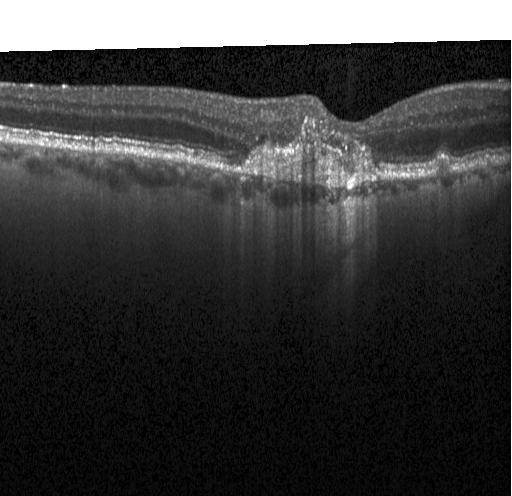 Retinal OCT B-scan, instrument: Heidelberg Spectralis, through the macula, spectral-domain optical coherence tomography
OCT finding: a choroidal neovascular membrane.